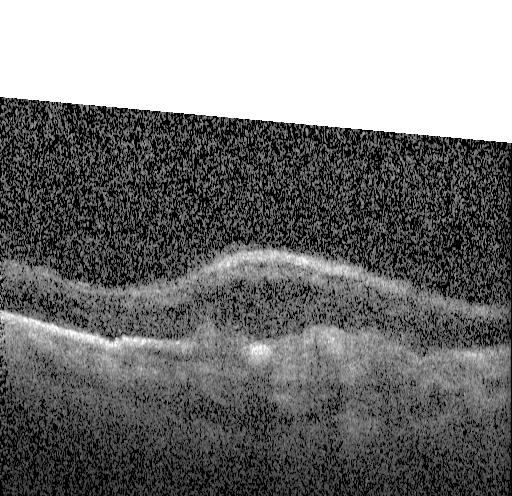 Finding: choroidal neovascularization (CNV).